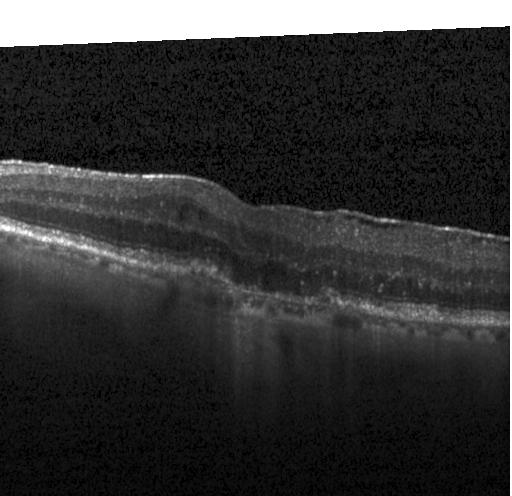

Optical coherence tomography B-scan, Heidelberg Spectralis OCT system, centered on the fovea, spectral-domain OCT
Finding: choroidal neovascularization (CNV).